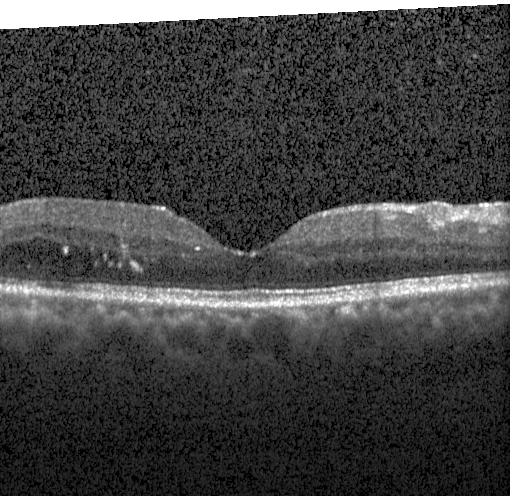
Horizontal scan through the fovea; OCT line scan; Heidelberg Spectralis. Finding: diabetic macular edema.